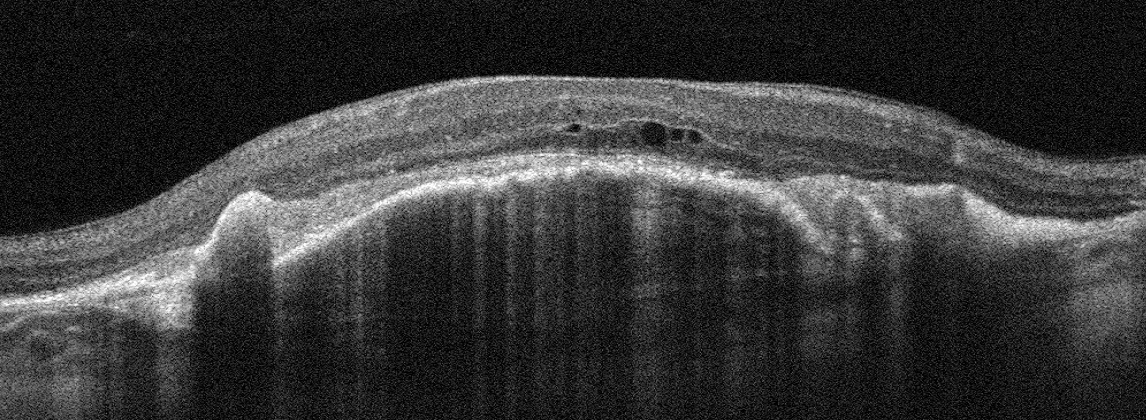

Macular OCT: AMD.